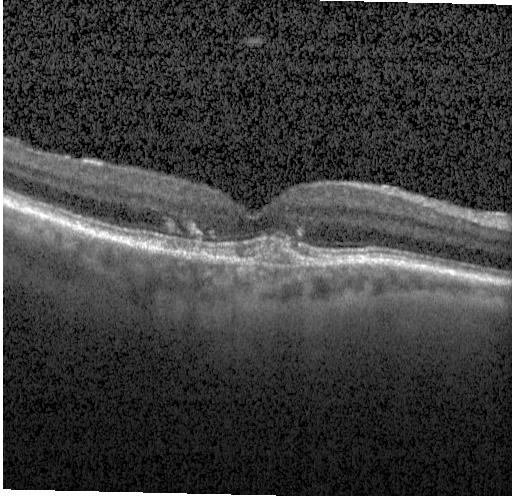
Instrument: Heidelberg Spectralis, OCT line scan
Finding: choroidal neovascularization.